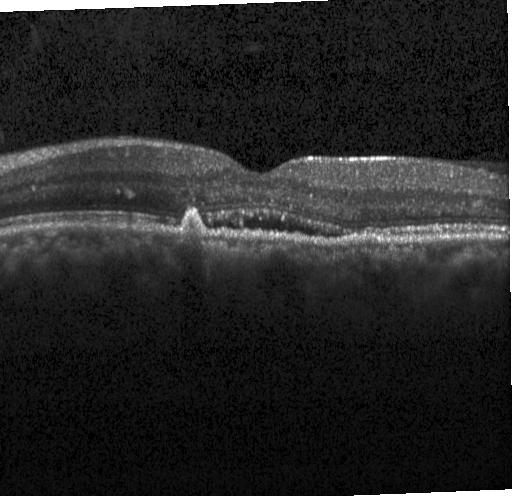
Impression: a choroidal neovascular membrane.